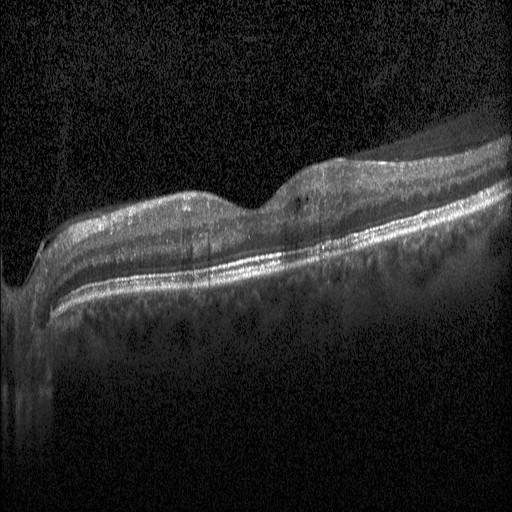

Optical coherence tomography scan; SD-OCT — Dx: diabetic macular edema (DME).